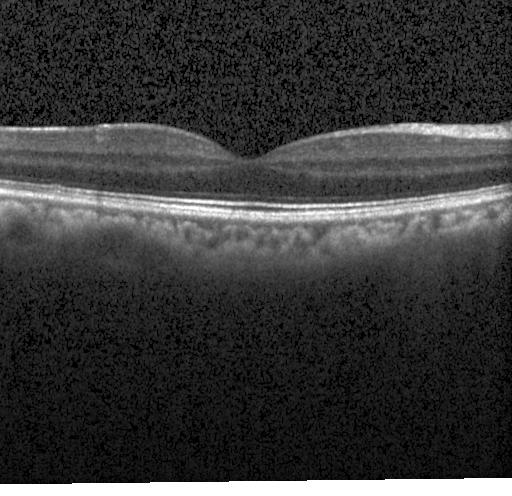

Assessment: neither CNV, DME, nor drusen.